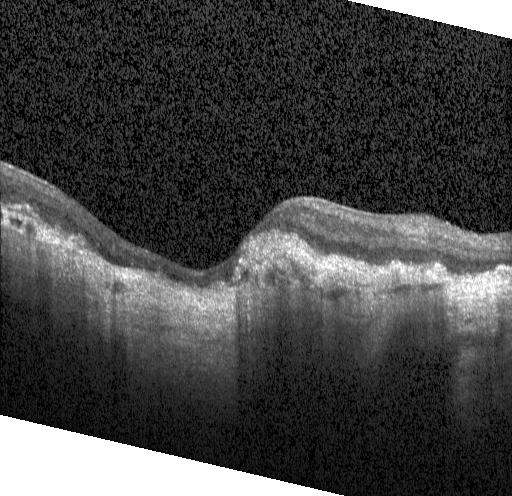

Finding: a choroidal neovascular membrane.